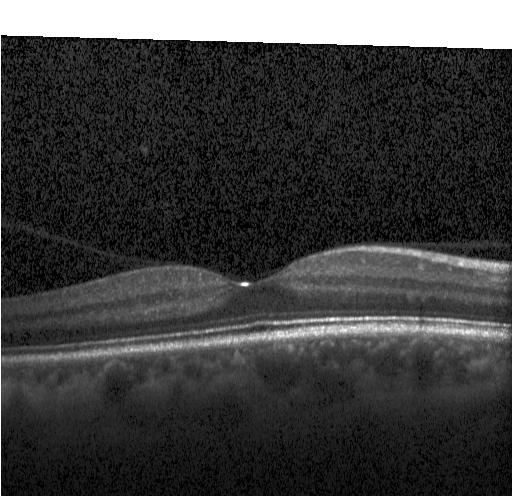
The scan shows no CNV, no DME, and no drusen.